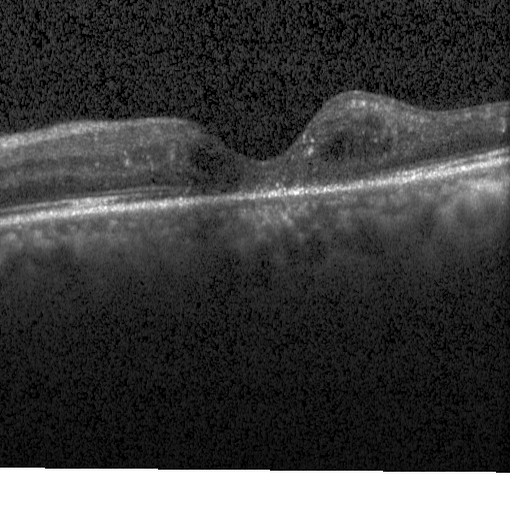
Spectral-domain optical coherence tomography; optical coherence tomography scan.
Diagnosis: DME.